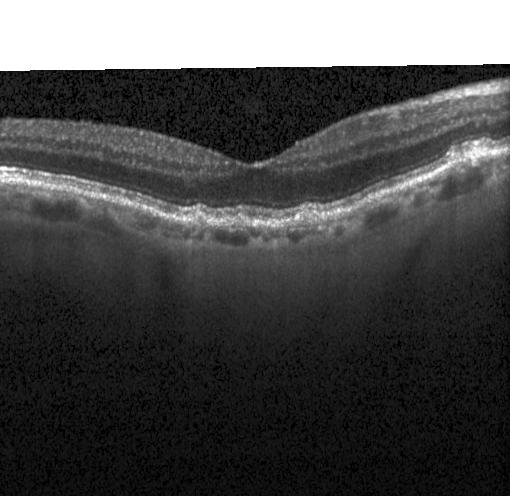
Optical coherence tomography B-scan
Macular OCT: sub-RPE drusenoid deposits.